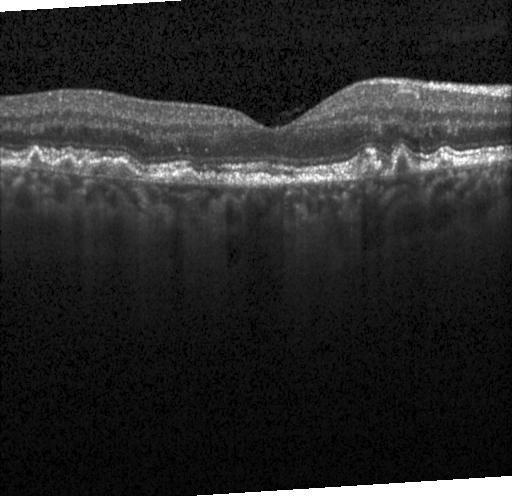
OCT scan showing drusen.